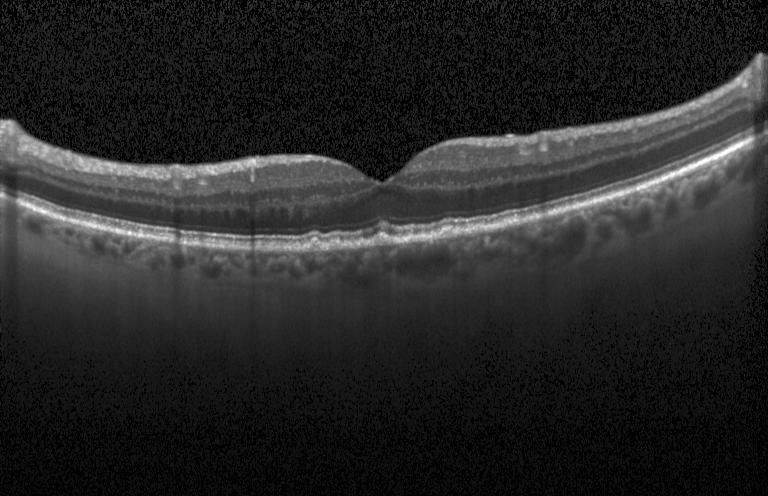 Macular OCT: multiple drusen.